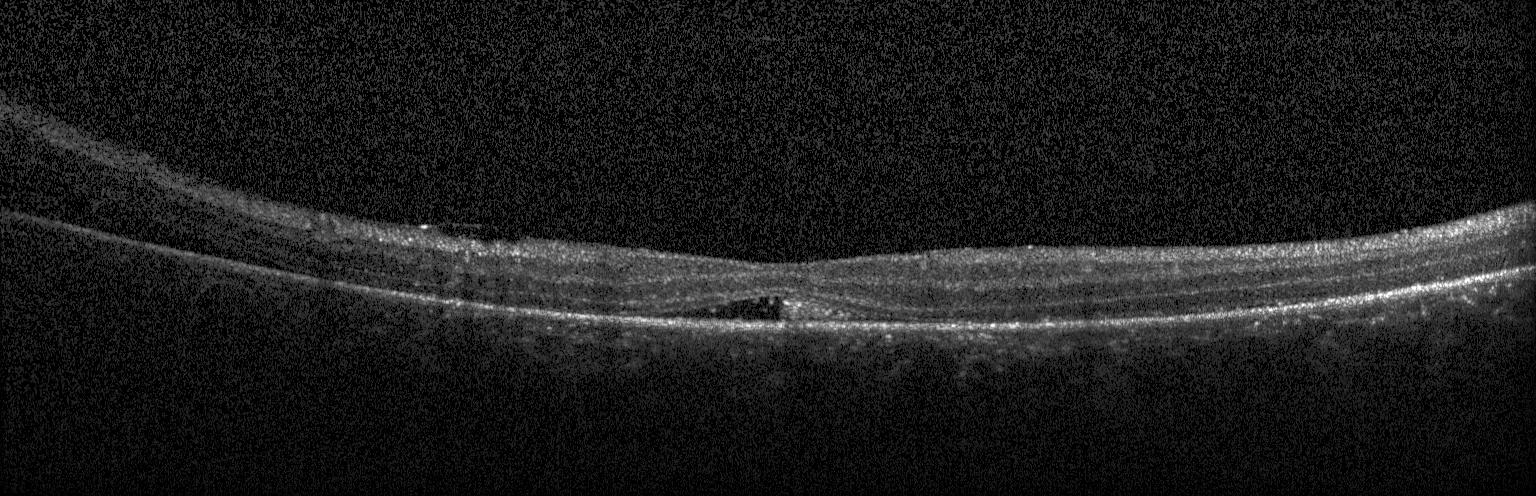

Fovea-centered. OCT line scan. Instrument: Heidelberg Spectralis
OCT finding: a choroidal neovascular membrane.